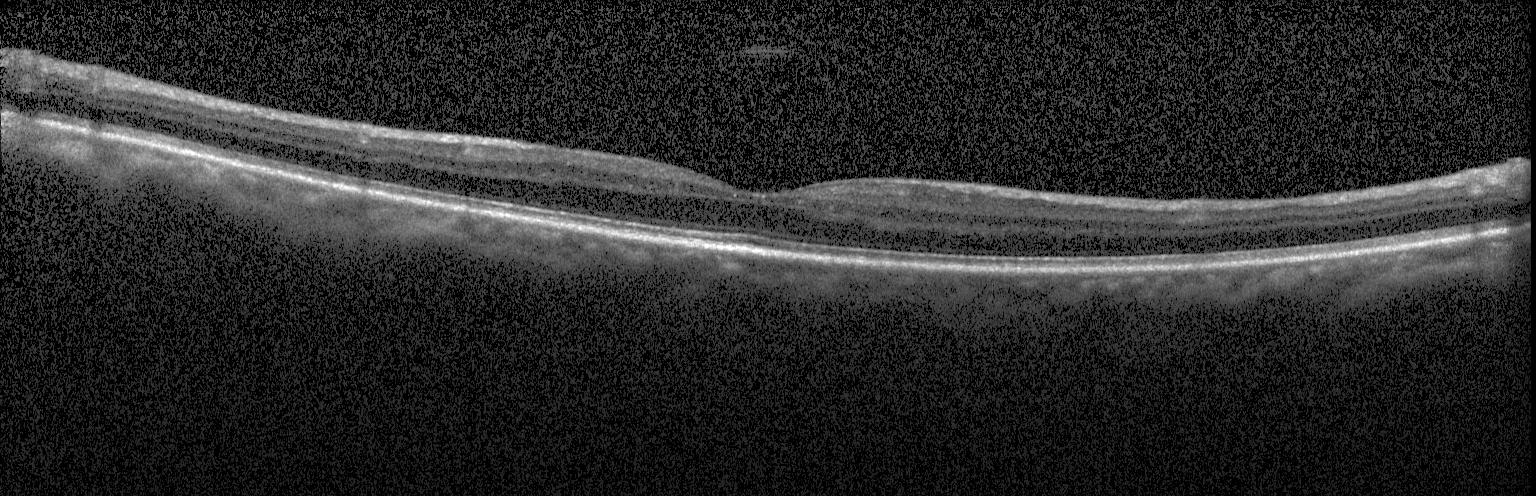 Optical coherence tomography scan. Neither CNV, DME, nor drusen.